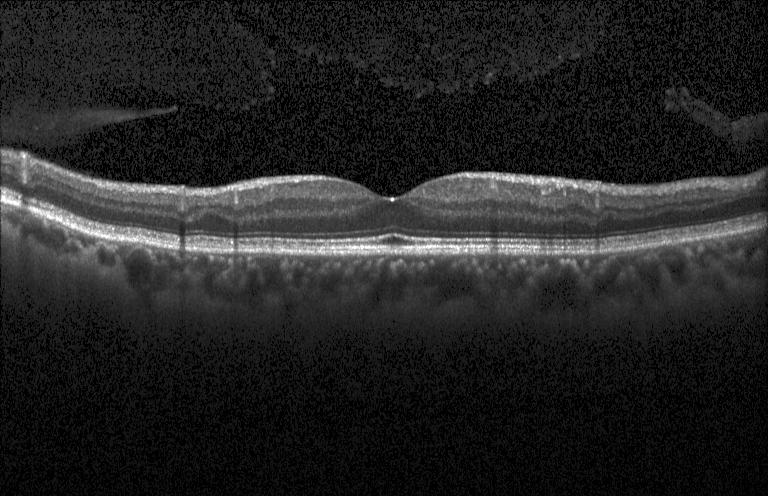 Retinal OCT cross-section, through the macula.
Finding: neither CNV, DME, nor drusen.